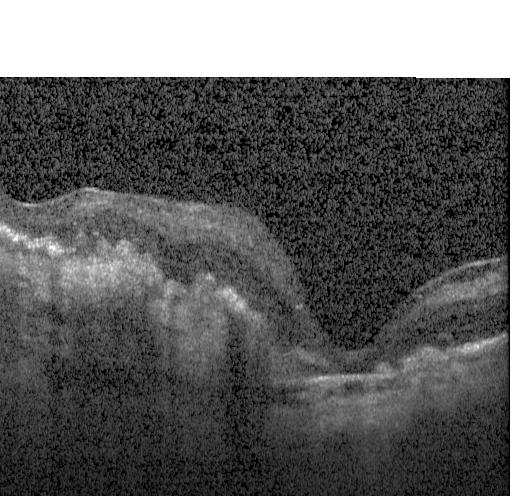

OCT line scan
Finding: choroidal neovascularization (CNV).